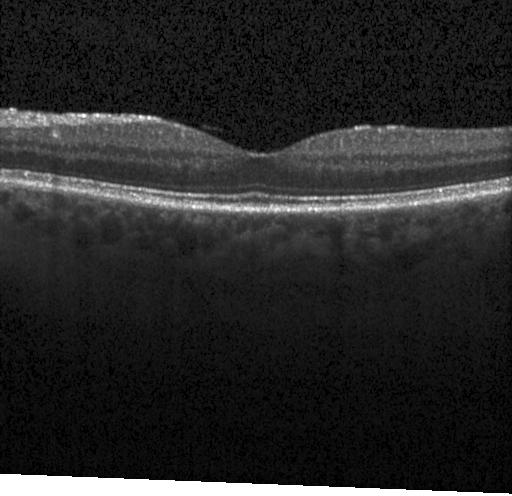
Impression: no choroidal neovascularization, diabetic macular edema, or drusen.